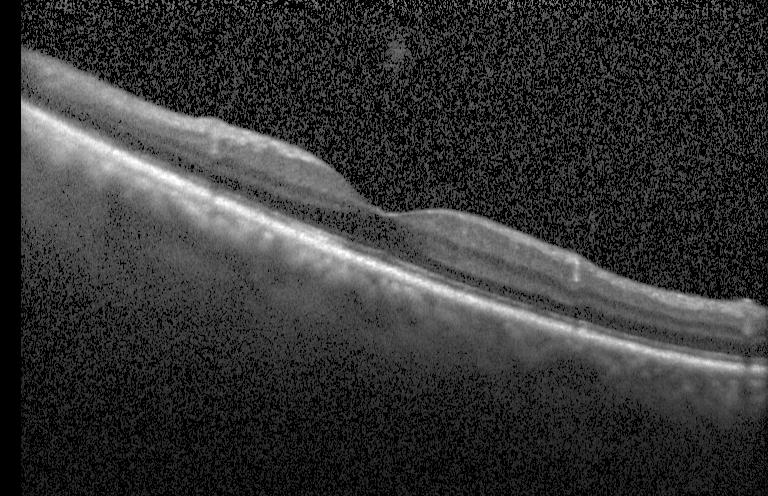 Spectral-domain optical coherence tomography. Acquired on a Heidelberg Spectralis. OCT B-scan. Impression: no choroidal neovascularization, diabetic macular edema, or drusen.